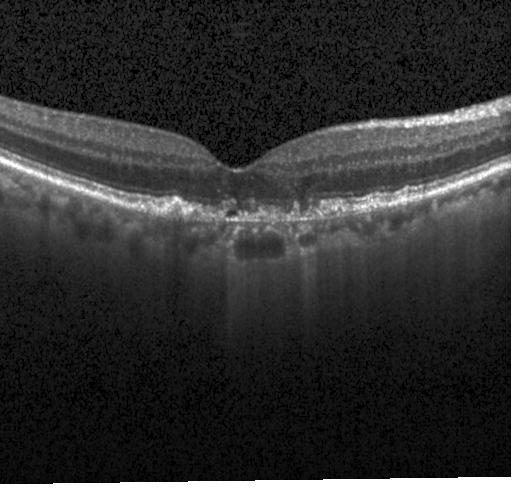
Retinal OCT cross-section, spectral-domain optical coherence tomography
The scan shows a choroidal neovascular membrane.